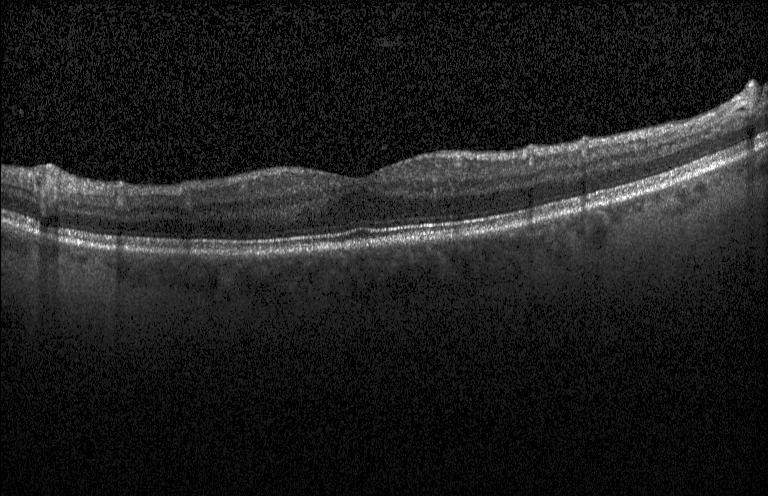

OCT B-scan
Finding: neither CNV, DME, nor drusen.